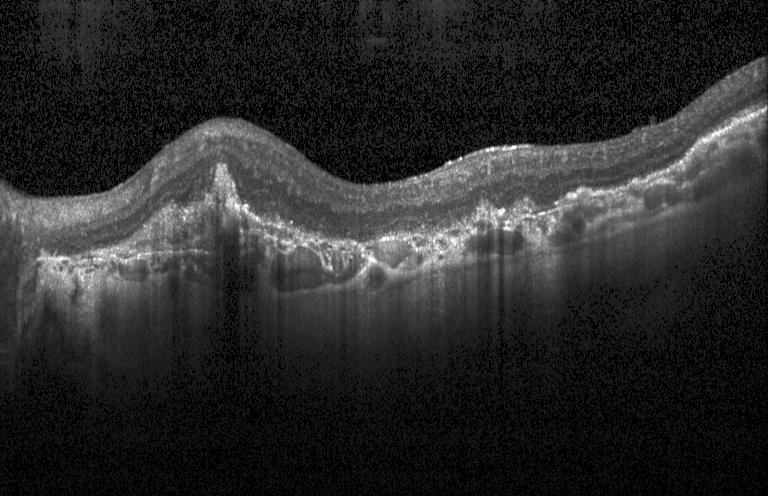 Centered on the fovea, OCT line scan, spectral-domain OCT — This B-scan demonstrates choroidal neovascularization (CNV).